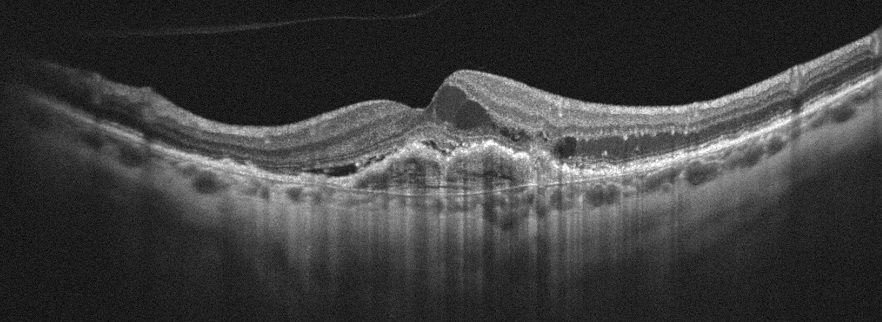

Impression: age-related macular degeneration (AMD).